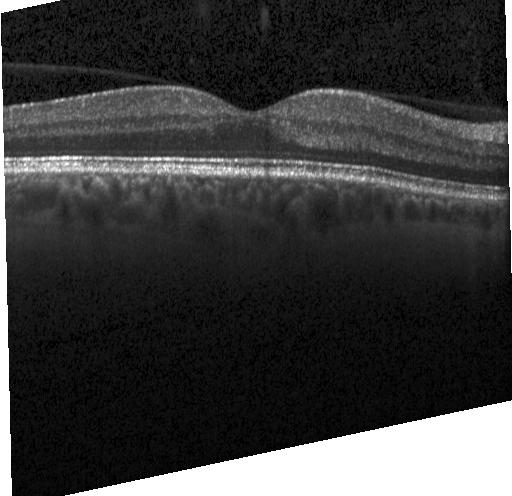

OCT B-scan showing no evidence of CNV, DME, or drusen.